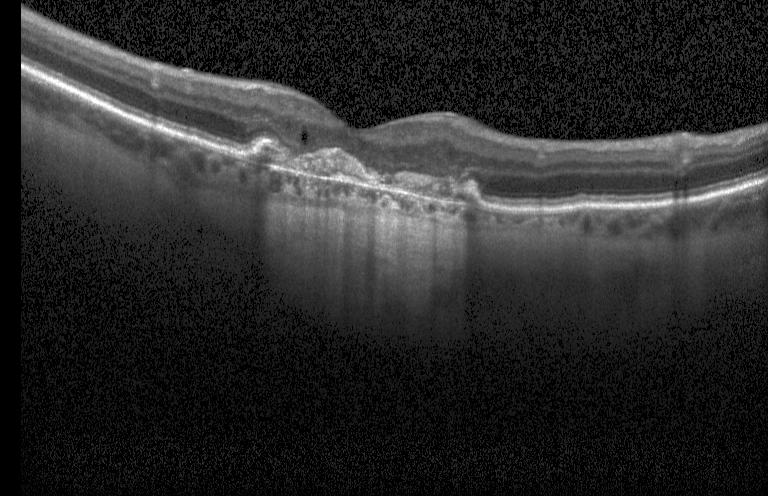
Retinal OCT cross-section — Diagnosis: a choroidal neovascular membrane.